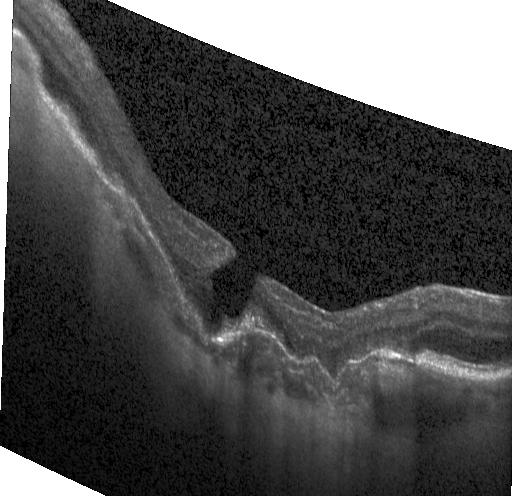 Instrument: Heidelberg Spectralis, SD-OCT, retinal OCT cross-section, fovea-centered
This B-scan demonstrates a choroidal neovascular membrane.